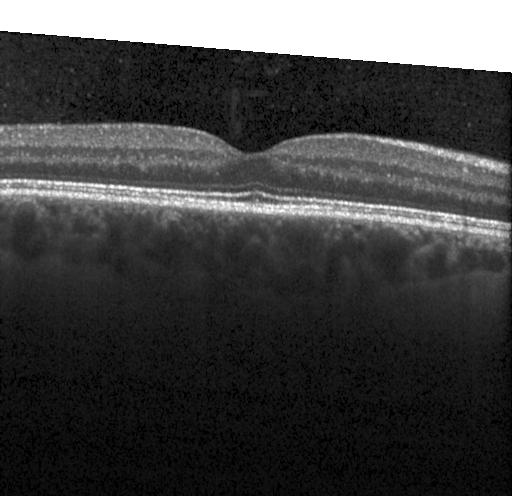
The scan shows no choroidal neovascularization, no diabetic macular edema, and no drusen.